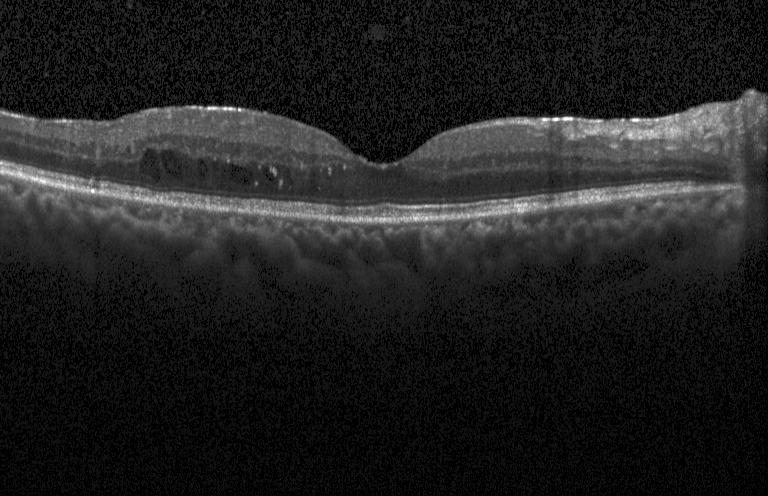 Instrument: Heidelberg Spectralis · optical coherence tomography B-scan · SD-OCT · macular scan.
Finding: DME.